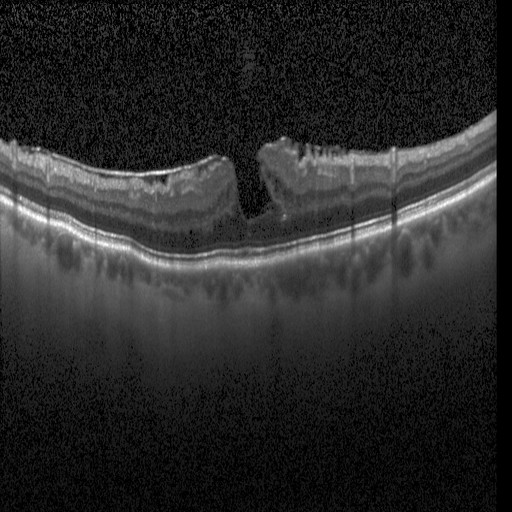

Retinal OCT cross-section — Impression: DME.